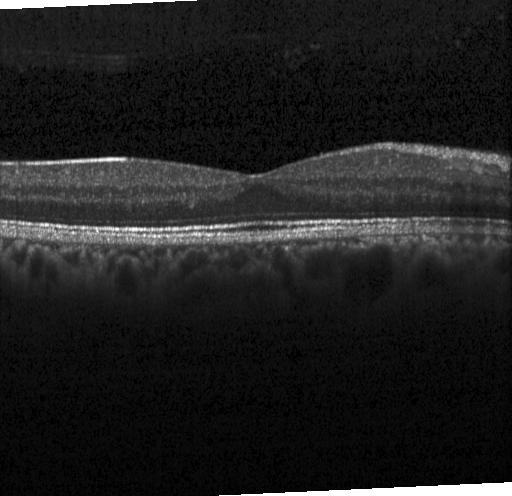
Retinal OCT cross-section showing no choroidal neovascularization, no diabetic macular edema, and no drusen.